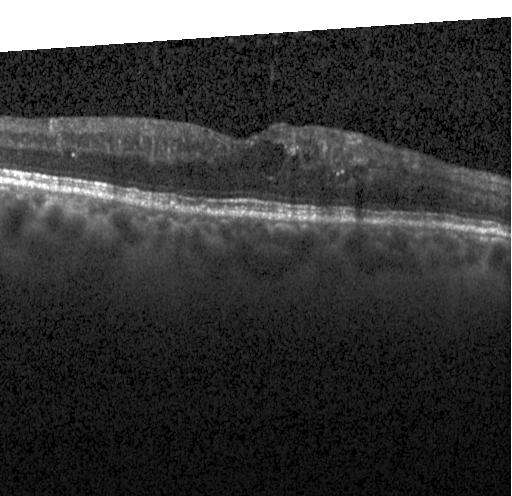 Diagnosis: diabetic macular edema (DME).